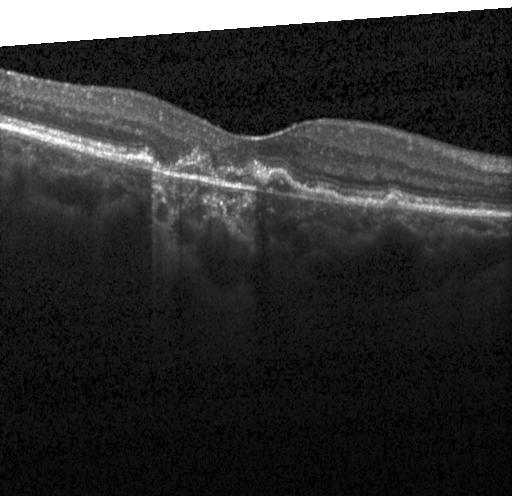

Finding: a choroidal neovascular membrane.